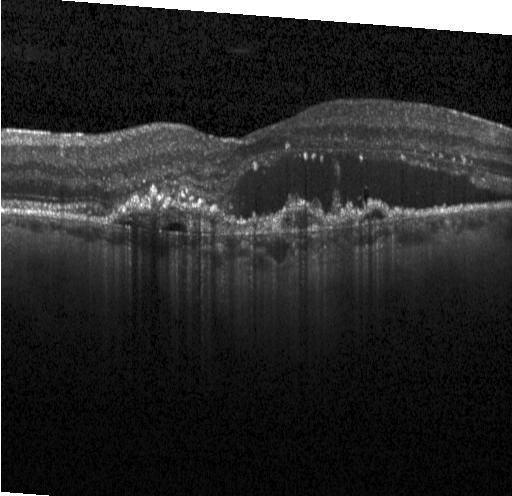 This B-scan demonstrates a choroidal neovascular membrane.